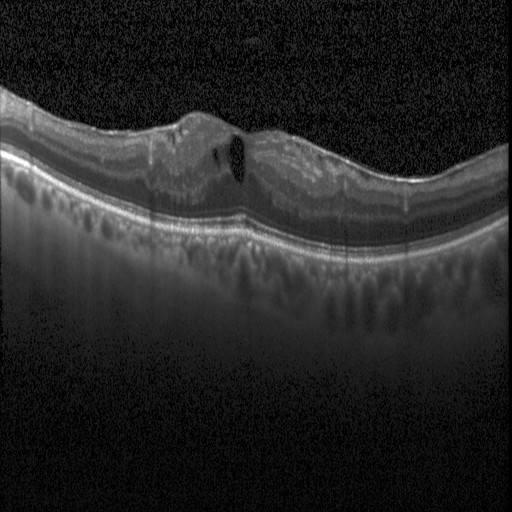 Optical coherence tomography scan; Heidelberg Spectralis OCT system; macular scan; SD-OCT. The scan shows DME.